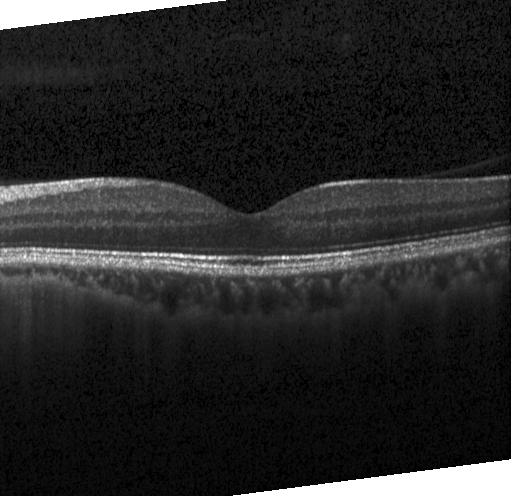

Impression: no choroidal neovascularization, diabetic macular edema, or drusen.